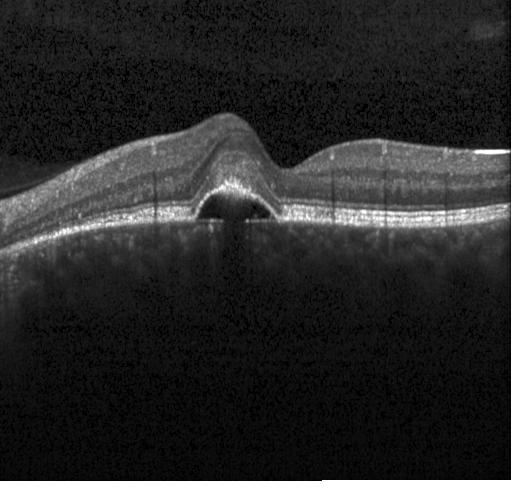 Spectral-domain optical coherence tomography · OCT line scan · macular scan.
This B-scan demonstrates a choroidal neovascular membrane.